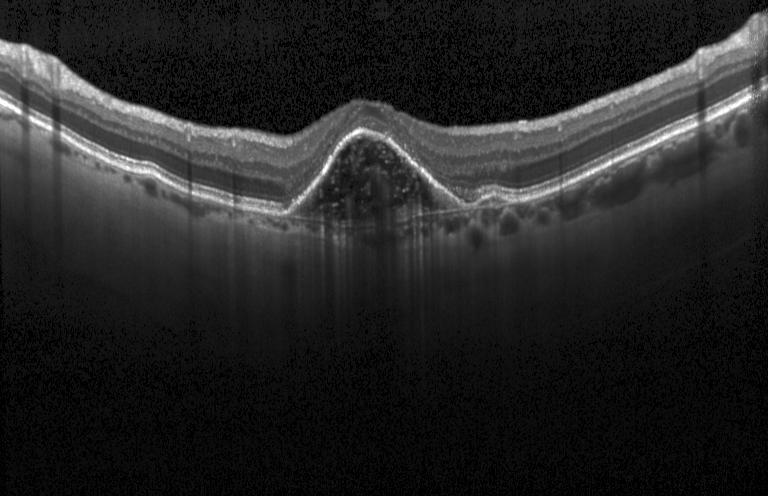 Finding: a choroidal neovascular membrane.